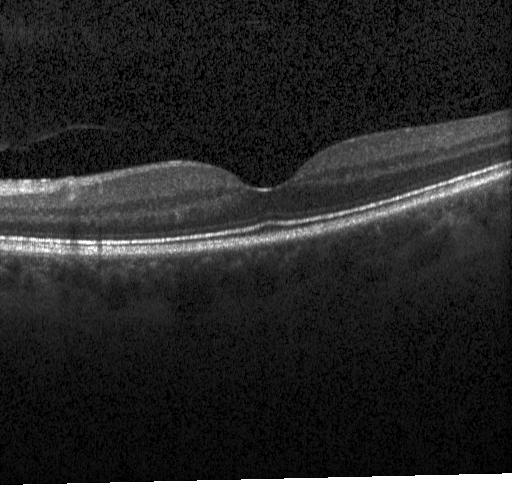
Retinal OCT cross-section — No CNV, DME, or drusen.